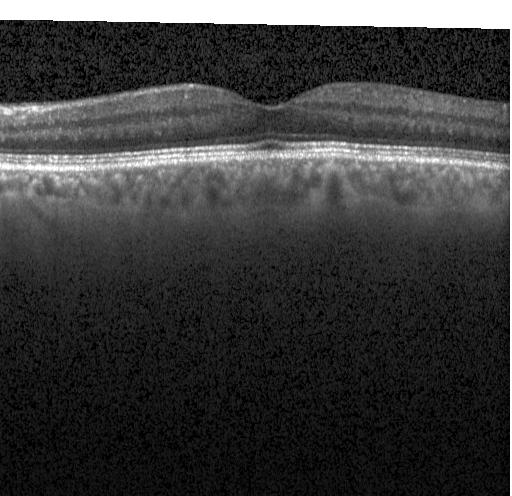 OCT B-scan. SD-OCT. Finding: no CNV, DME, or drusen.